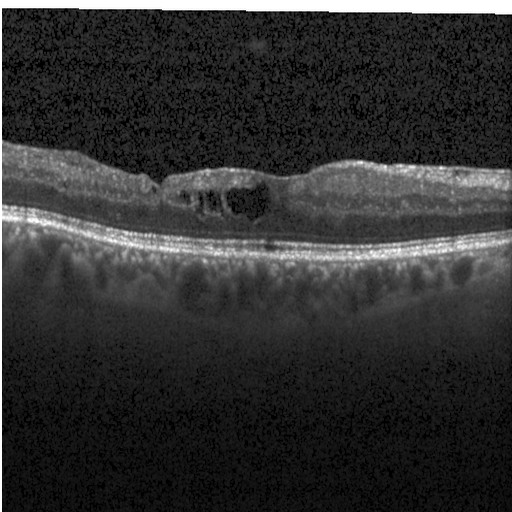

SD-OCT; retinal OCT B-scan
Diabetic macular edema (DME).